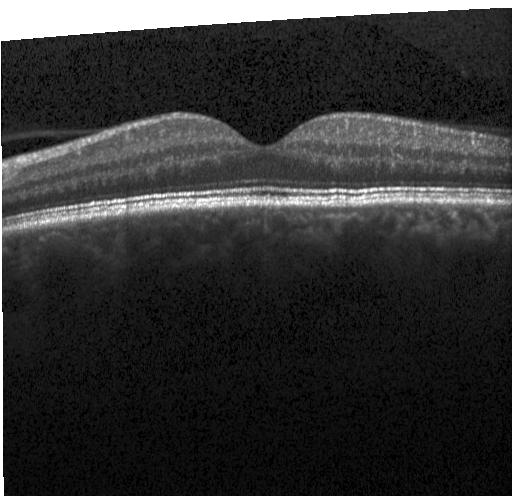

Spectral-domain OCT B-scan: no evidence of CNV, DME, or drusen.